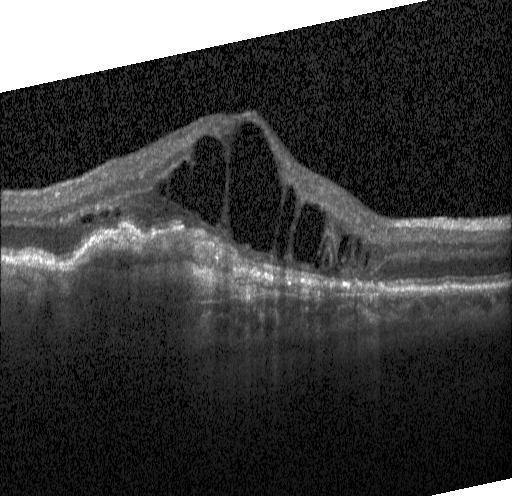

Macular OCT: a choroidal neovascular membrane.